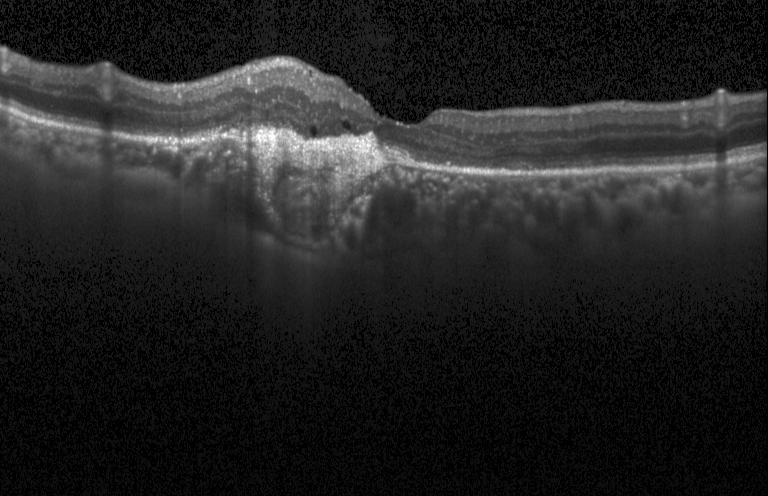

Retinal OCT cross-section showing CNV.